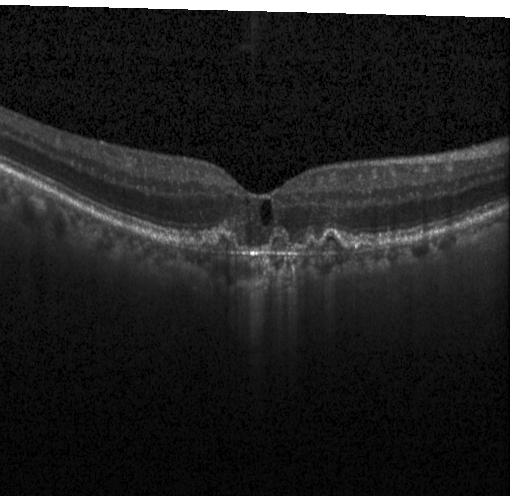
Finding: choroidal neovascularization.